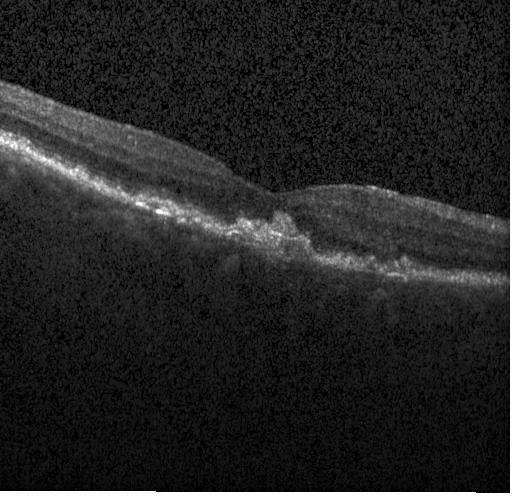 Impression: choroidal neovascularization.